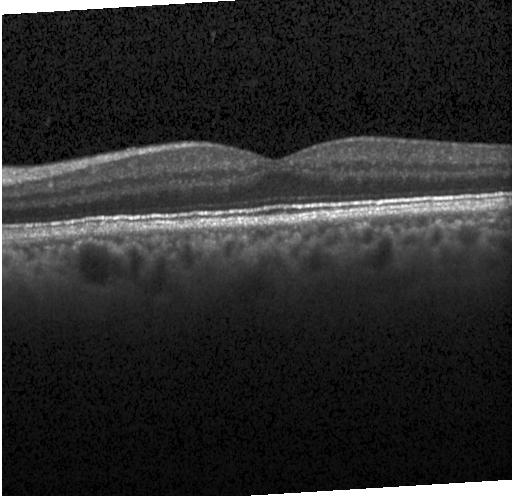 Retinal OCT cross-section; centered on the fovea; spectral-domain OCT
This B-scan demonstrates neither choroidal neovascularization, diabetic macular edema, nor drusen.